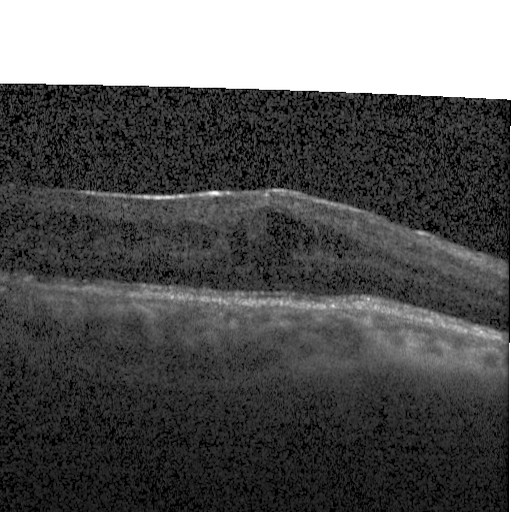
Heidelberg Spectralis, SD-OCT, macular scan, retinal OCT B-scan
Diagnosis: diabetic macular edema.